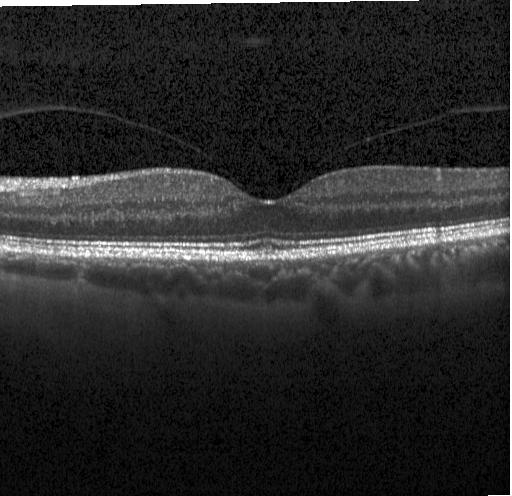

Optical coherence tomography scan, fovea-centered, spectral-domain optical coherence tomography. Impression: no choroidal neovascularization, no diabetic macular edema, and no drusen.